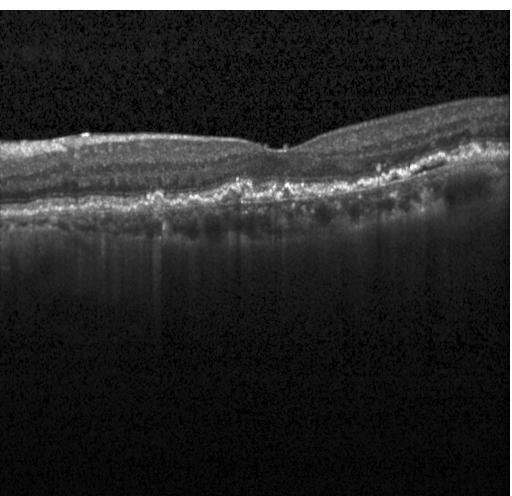

Retinal OCT B-scan. OCT finding: choroidal neovascularization.